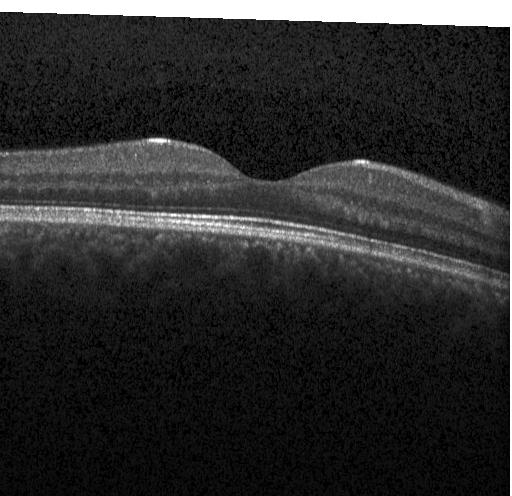

Retinal OCT cross-section showing no evidence of choroidal neovascularization, diabetic macular edema, or drusen.